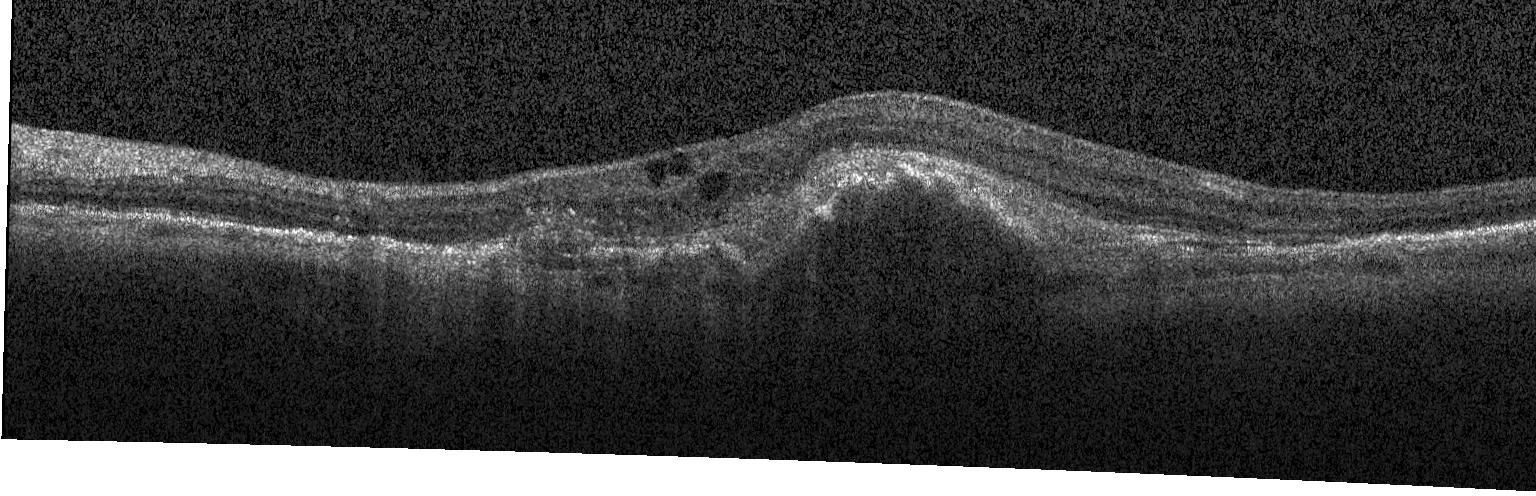 OCT line scan. Macular scan. Spectral-domain OCT
Dx: a choroidal neovascular membrane.